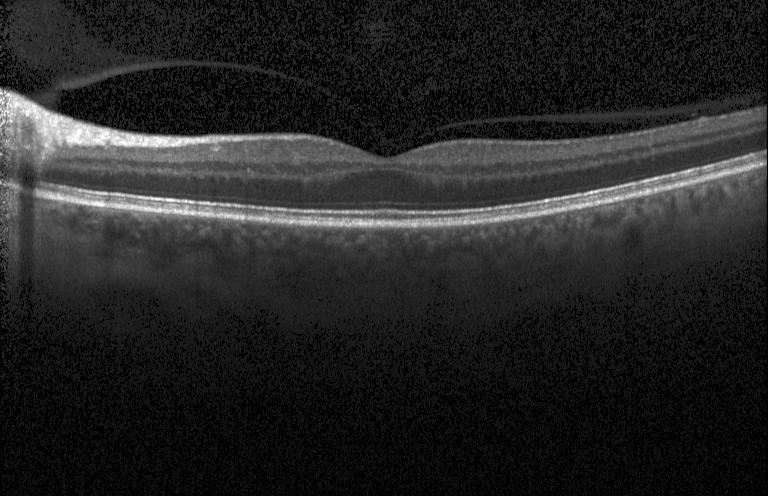

Spectral-domain OCT B-scan: no CNV, no DME, and no drusen.